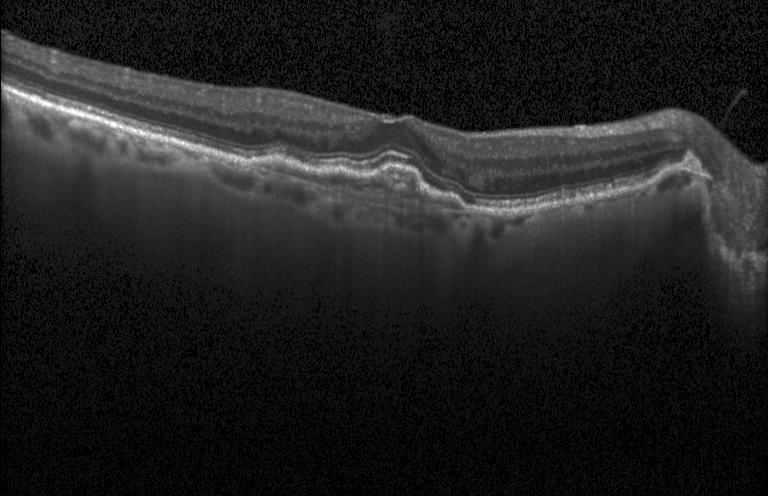

Instrument: Heidelberg Spectralis, spectral-domain OCT, horizontal scan through the fovea, retinal OCT B-scan — Impression: a choroidal neovascular membrane.